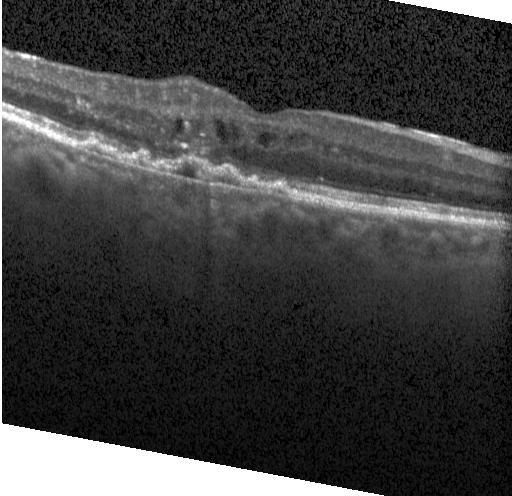 OCT line scan · Heidelberg Spectralis OCT system · fovea-centered · SD-OCT. Diagnosis: choroidal neovascularization (CNV).